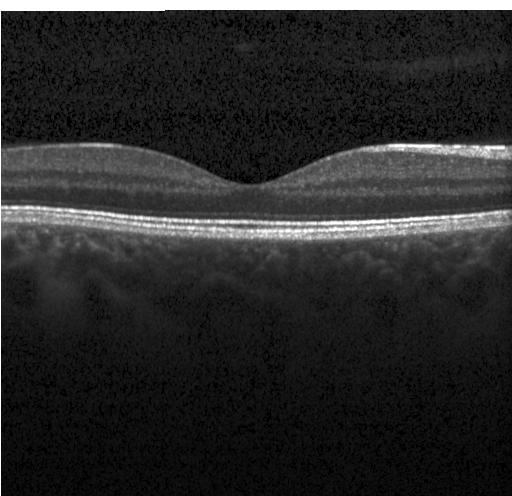
Instrument: Heidelberg Spectralis · optical coherence tomography scan
The scan shows no choroidal neovascularization, diabetic macular edema, or drusen.